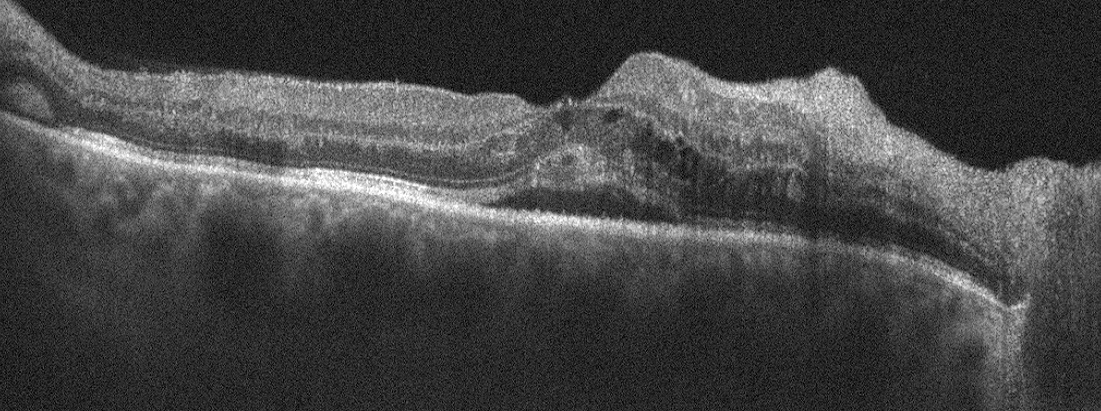

Diagnosis: RVO.